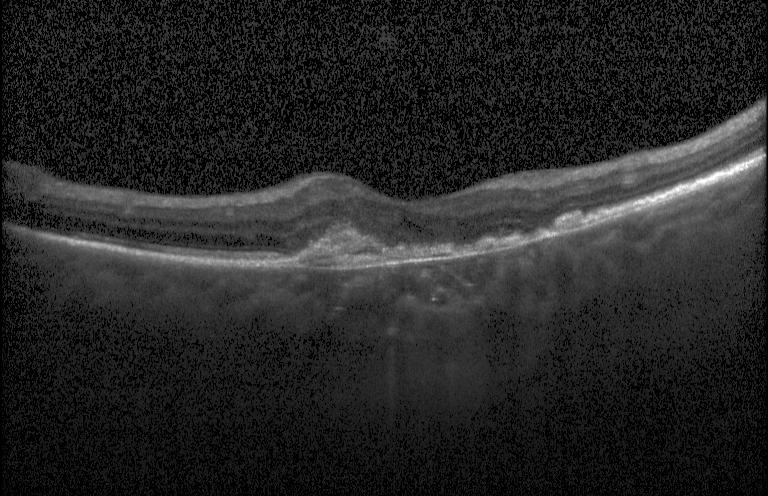 Heidelberg Spectralis OCT system; optical coherence tomography scan
Diagnosis: a choroidal neovascular membrane.